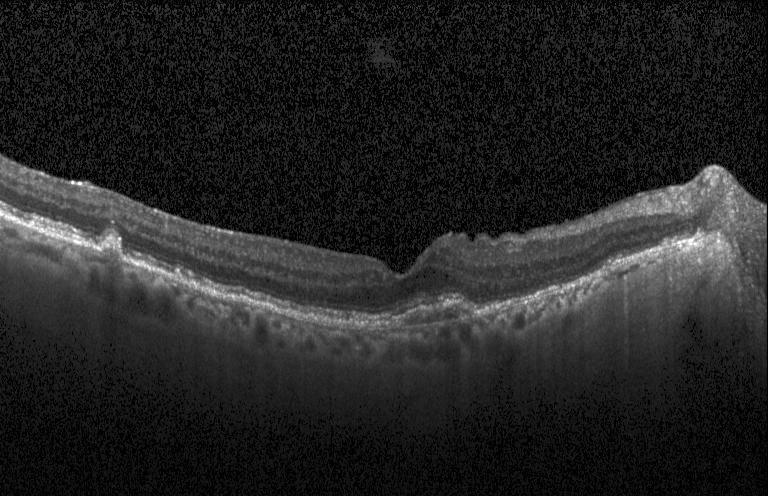
Retinal OCT B-scan.
The scan shows a choroidal neovascular membrane.